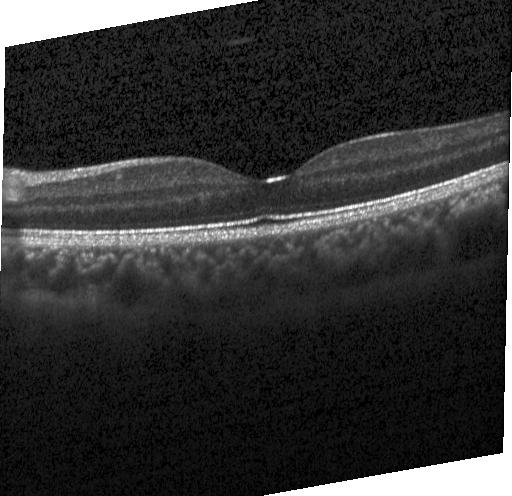

OCT B-scan
Diagnosis: no evidence of choroidal neovascularization, diabetic macular edema, or drusen.